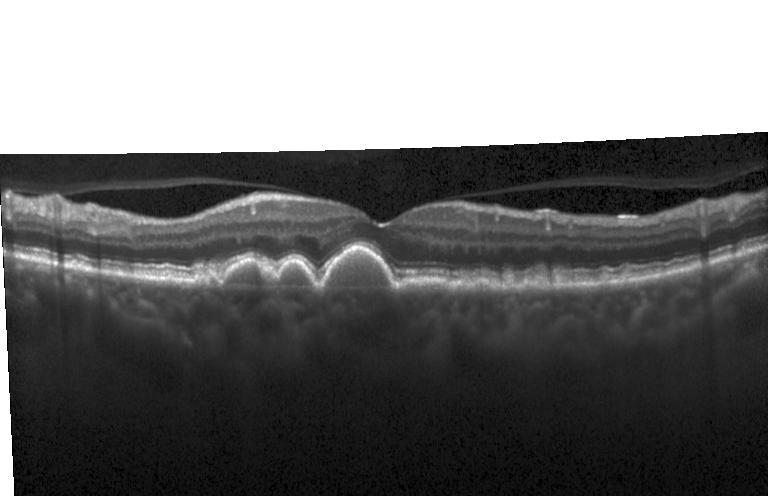 Retinal OCT cross-section showing drusen.